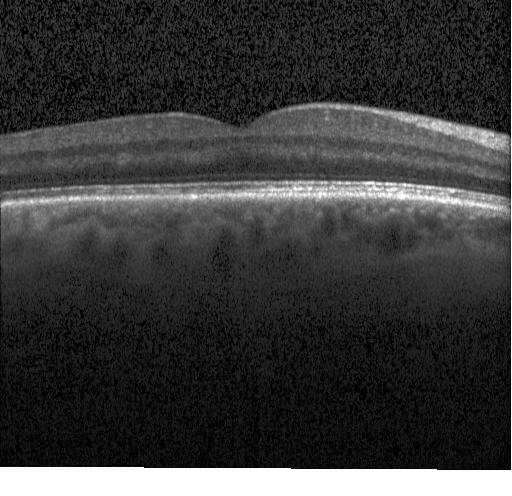
Optical coherence tomography B-scan · macular scan · Heidelberg Spectralis · spectral-domain OCT — Dx: neither choroidal neovascularization, diabetic macular edema, nor drusen.